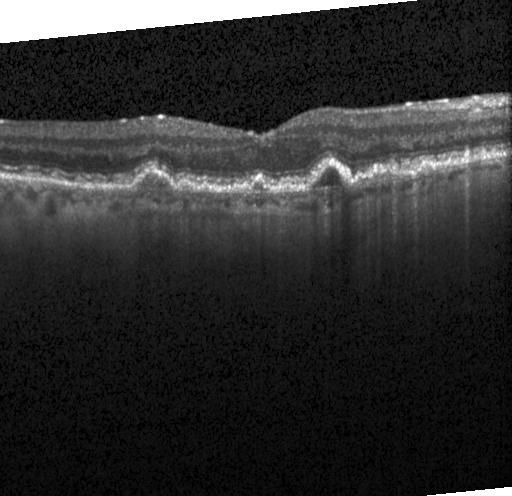
Retinal OCT B-scan. The scan shows CNV.